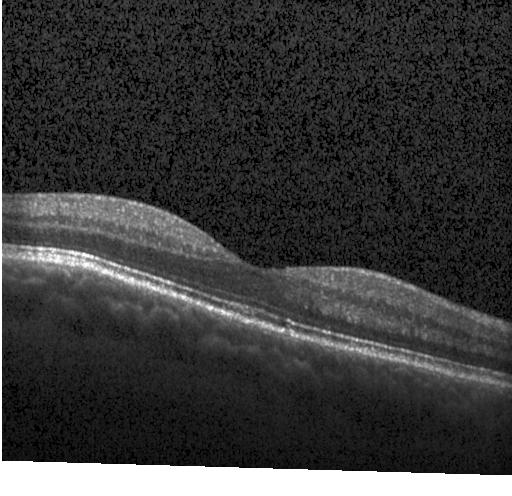

Instrument: Heidelberg Spectralis; optical coherence tomography scan
Diagnosis: no CNV, no DME, and no drusen.